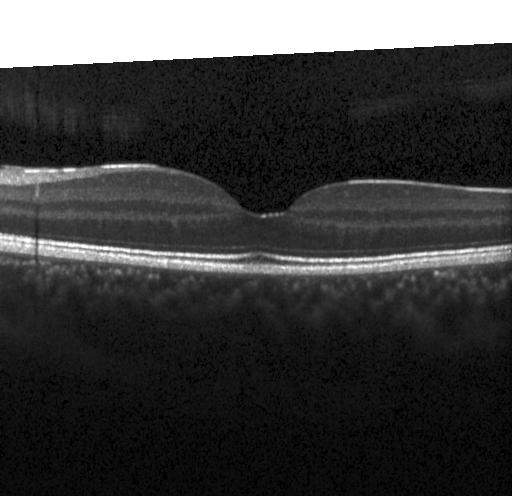
OCT line scan, acquired on a Heidelberg Spectralis, centered on the fovea, spectral-domain optical coherence tomography. This B-scan demonstrates no CNV, no DME, and no drusen.